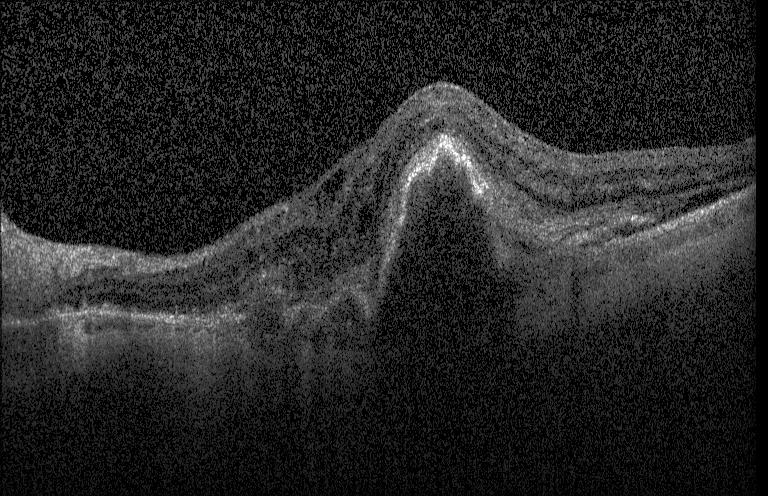

Impression: a choroidal neovascular membrane.